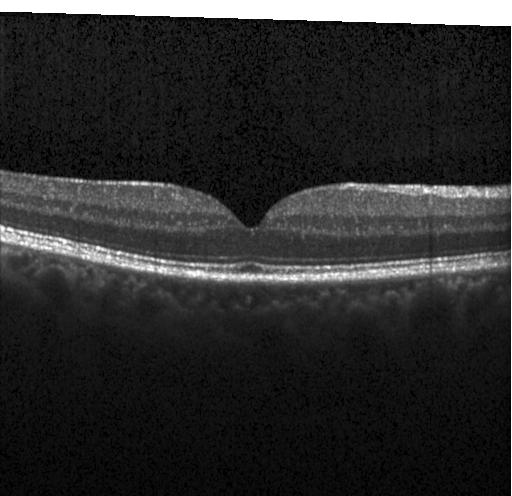
Retinal OCT B-scan — Finding: no evidence of choroidal neovascularization, diabetic macular edema, or drusen.